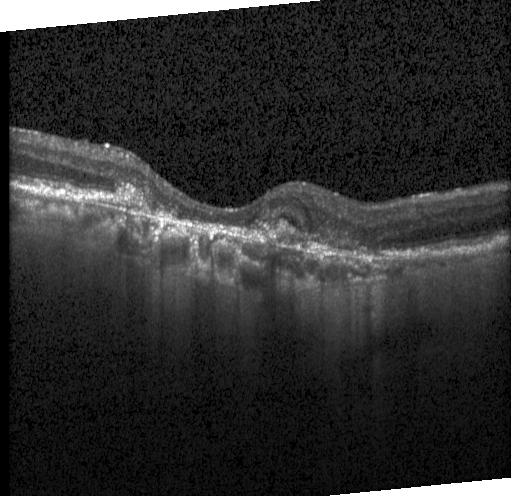
Heidelberg Spectralis OCT system. Optical coherence tomography scan. Through the macula
Diagnosis: choroidal neovascularization.